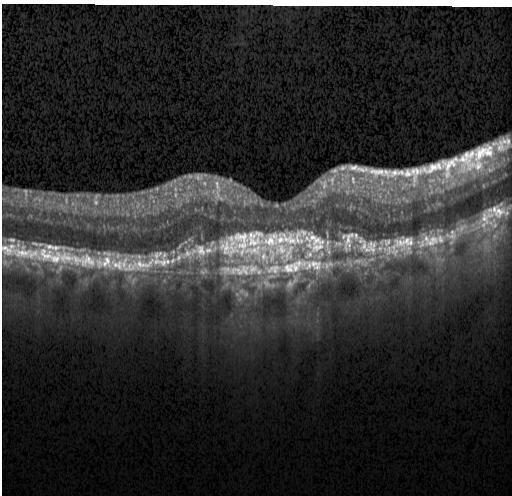 Diagnosis: CNV.